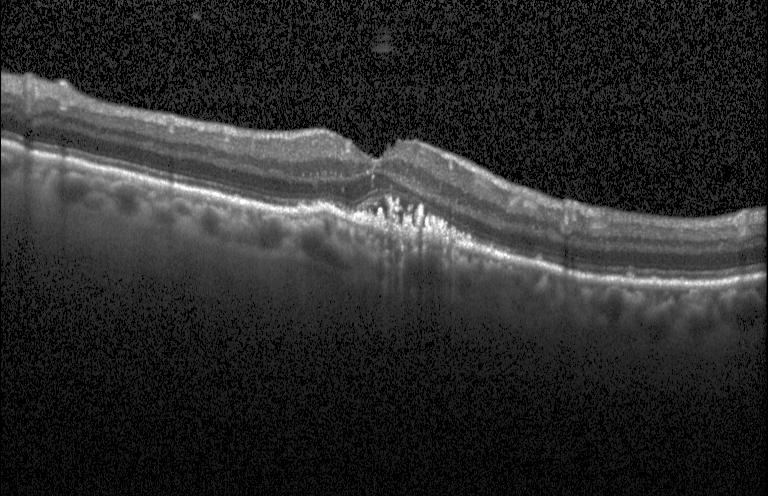

Impression: CNV.